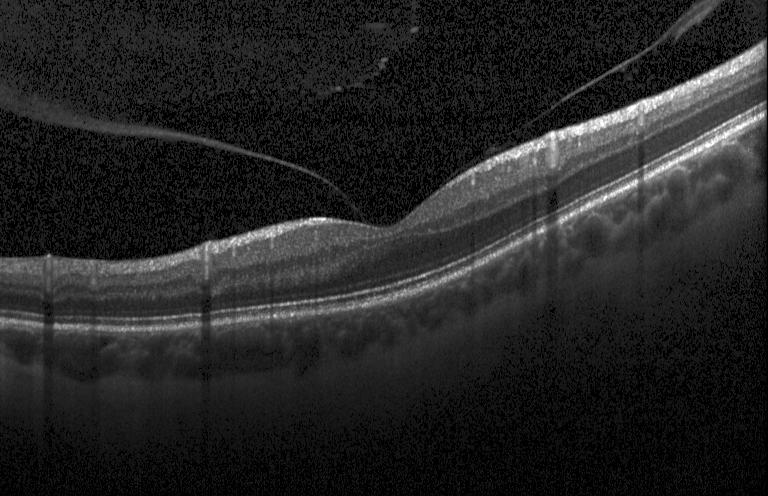
Neither CNV, DME, nor drusen.